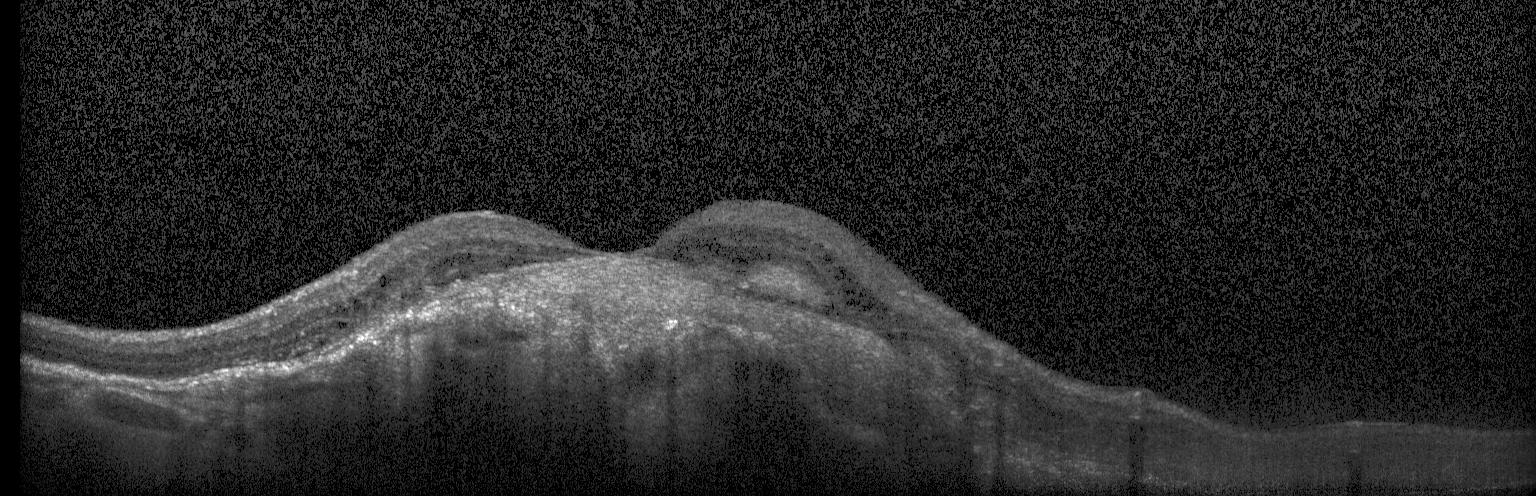 Centered on the fovea, optical coherence tomography B-scan — Macular OCT: a choroidal neovascular membrane.